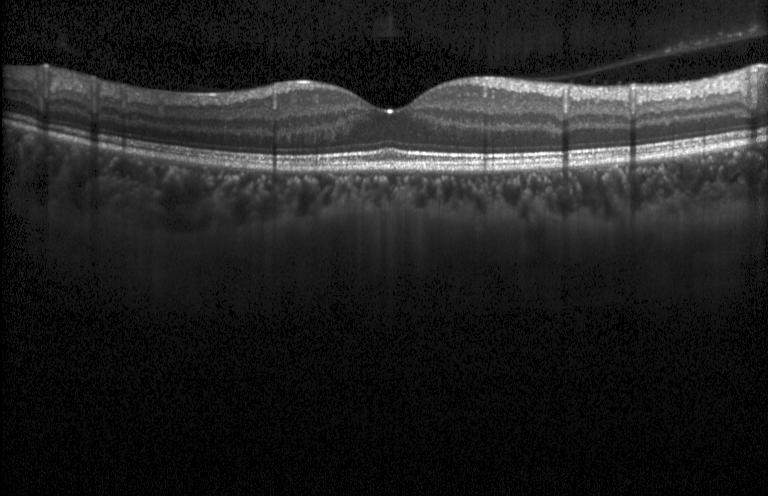
OCT line scan; SD-OCT; Heidelberg Spectralis OCT system. OCT finding: no CNV, no DME, and no drusen.